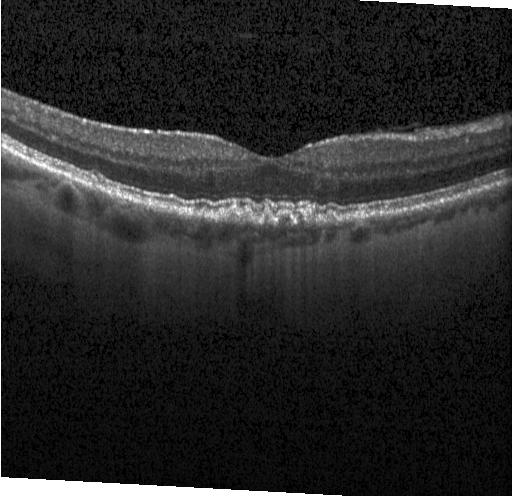
OCT line scan.
Assessment: sub-RPE drusenoid deposits.